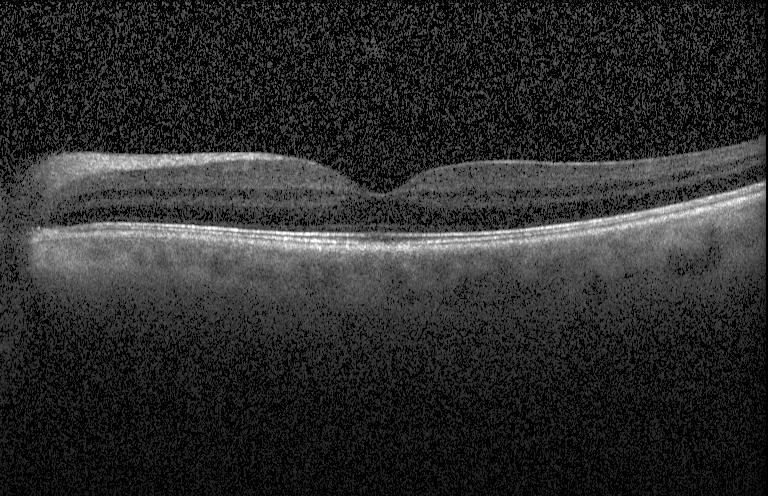
Impression: neither choroidal neovascularization, diabetic macular edema, nor drusen.